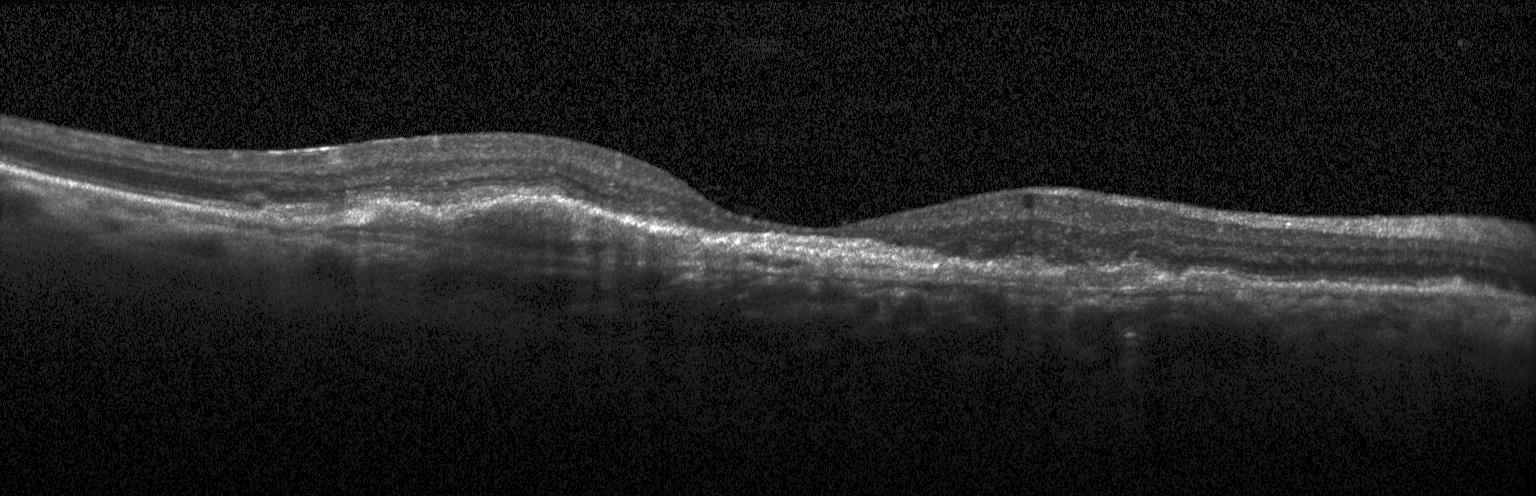

Optical coherence tomography B-scan; instrument: Heidelberg Spectralis; macular scan; spectral-domain optical coherence tomography
Finding: a choroidal neovascular membrane.